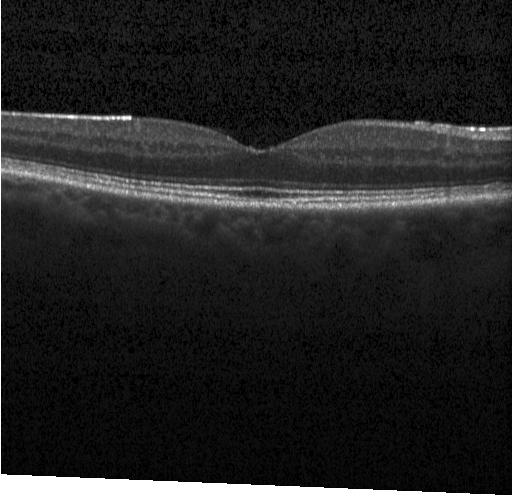

OCT line scan — Impression: no choroidal neovascularization, no diabetic macular edema, and no drusen.